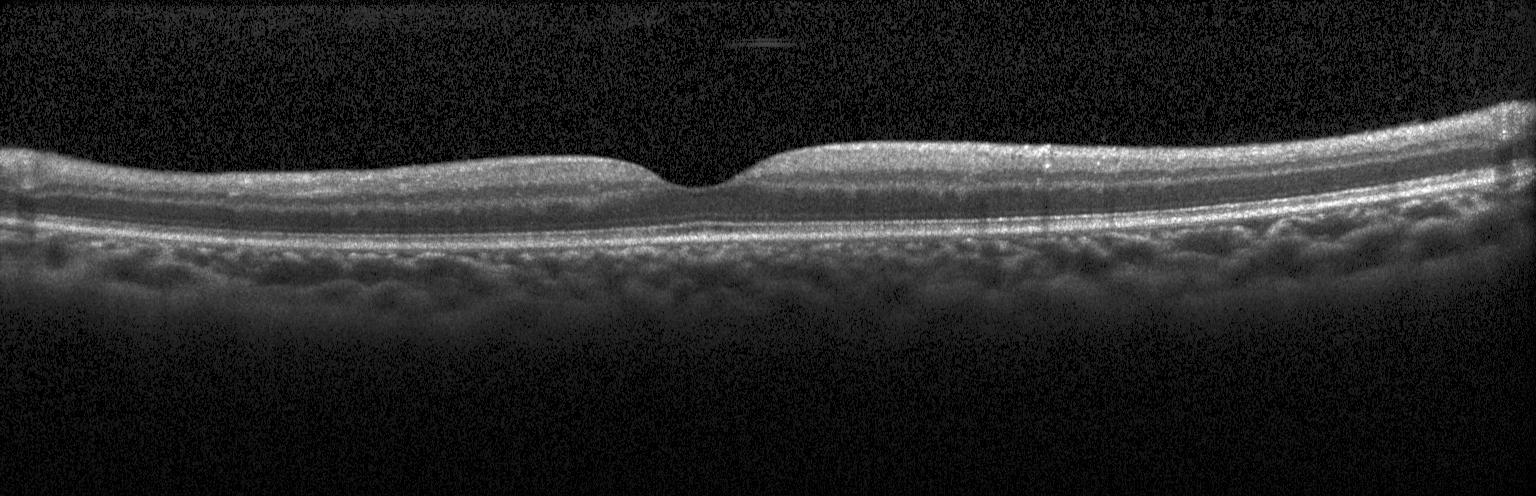

Horizontal scan through the fovea. OCT line scan. Instrument: Heidelberg Spectralis. Impression: neither choroidal neovascularization, diabetic macular edema, nor drusen.